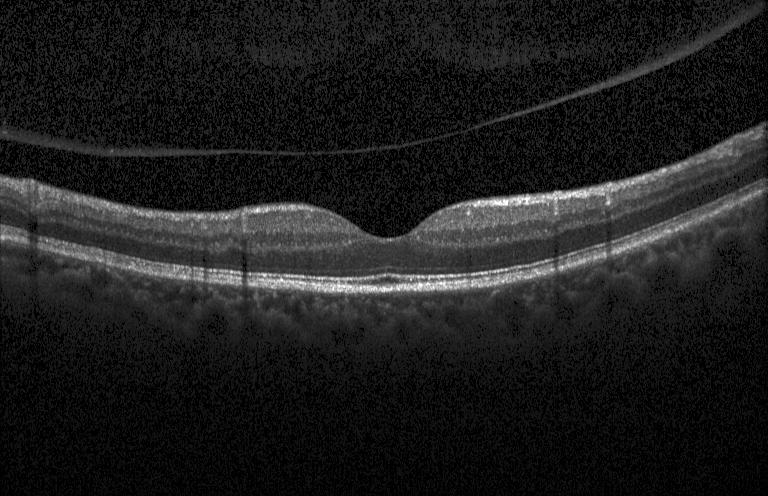

Impression: neither choroidal neovascularization, diabetic macular edema, nor drusen.